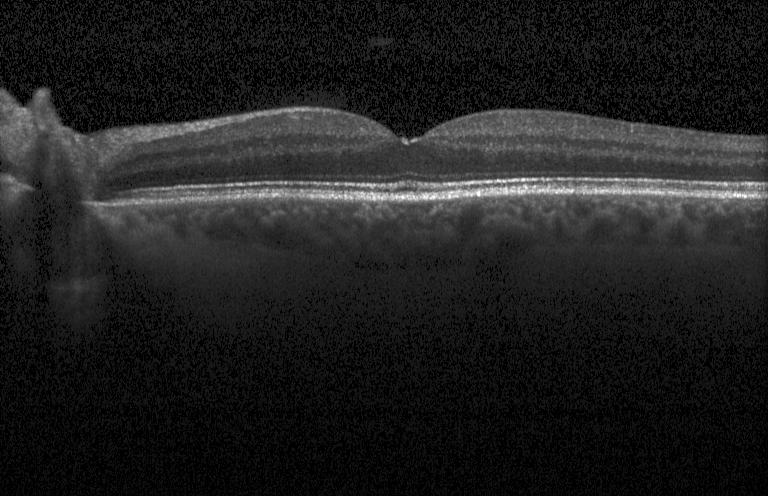

OCT scan showing no CNV, DME, or drusen.